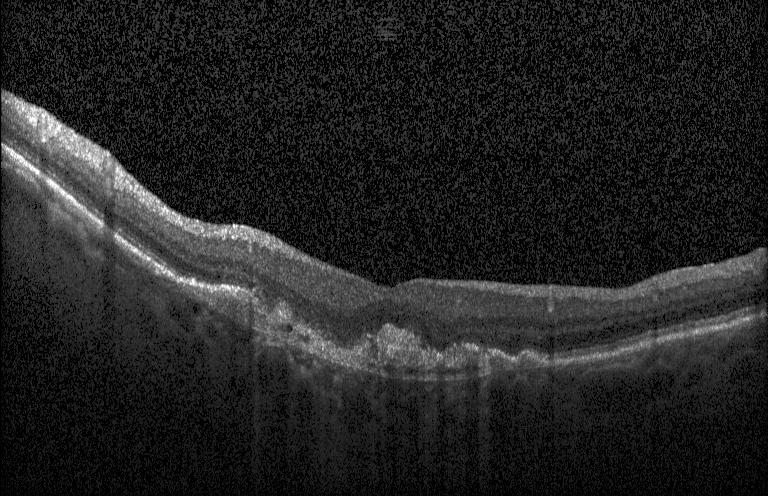 Heidelberg Spectralis OCT system · fovea-centered · OCT line scan — Dx: choroidal neovascularization (CNV).